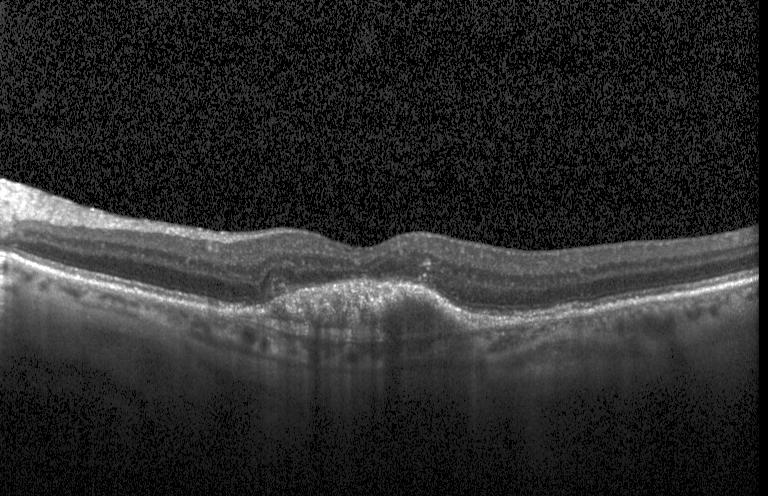
Finding: choroidal neovascularization.